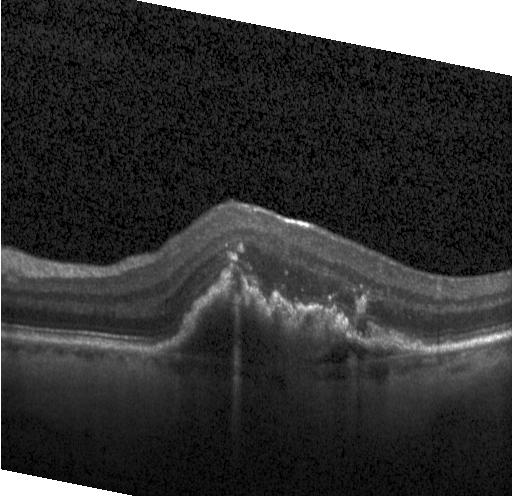 Impression: choroidal neovascularization.